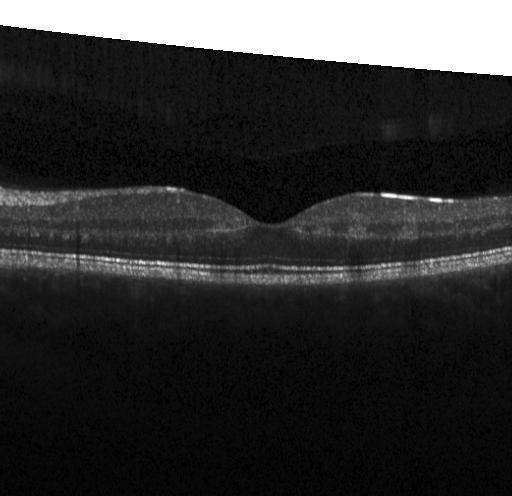
This B-scan demonstrates neither CNV, DME, nor drusen.